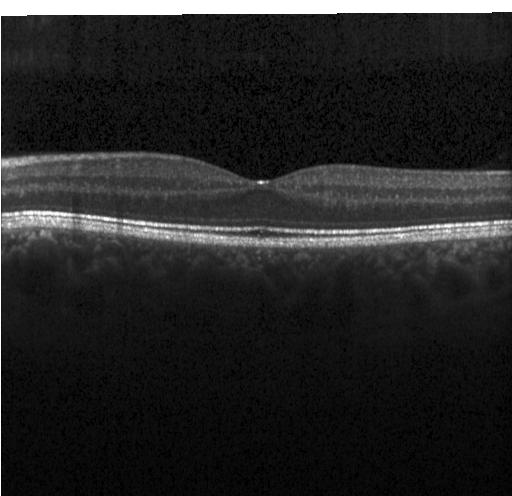 Centered on the fovea; SD-OCT; Heidelberg Spectralis OCT system; OCT line scan
Impression: no choroidal neovascularization, diabetic macular edema, or drusen.